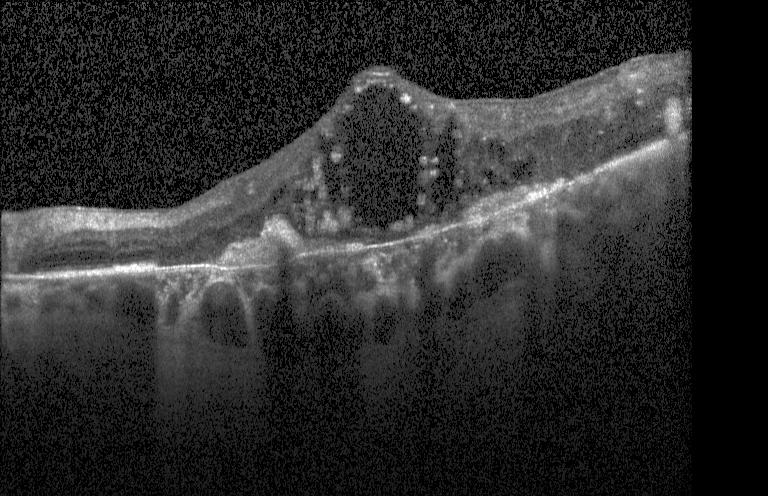

Retinal OCT cross-section, through the macula. Impression: CNV.